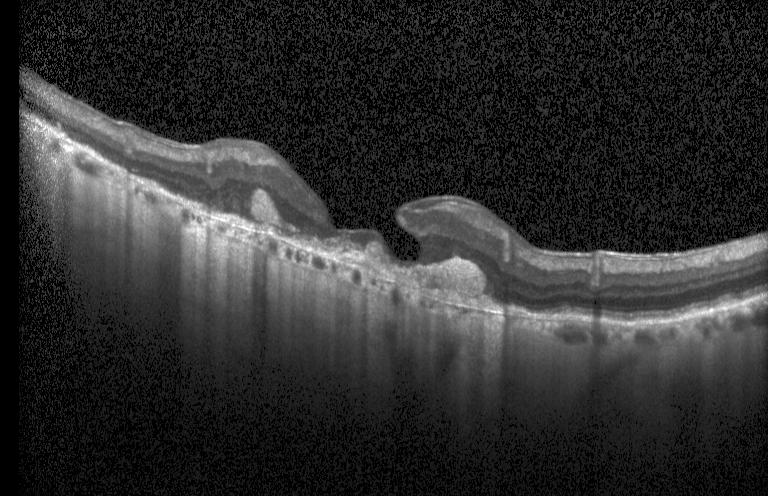

Macular scan, retinal OCT B-scan
Impression: choroidal neovascularization (CNV).